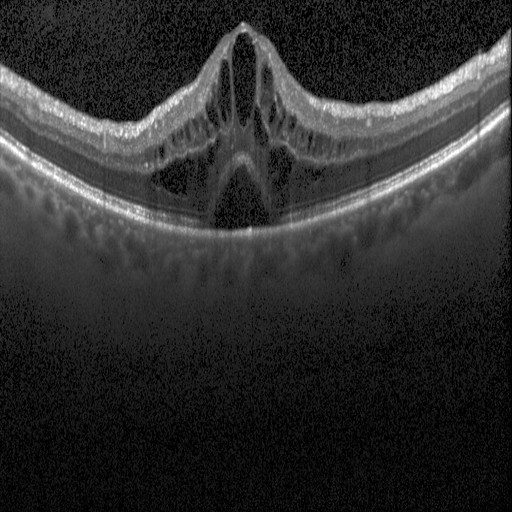
Spectral-domain OCT. OCT line scan — Assessment: diabetic macular edema (DME).